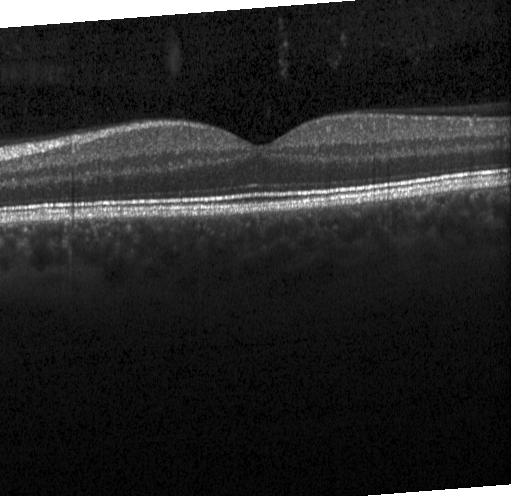

Optical coherence tomography scan.
The scan shows no CNV, DME, or drusen.